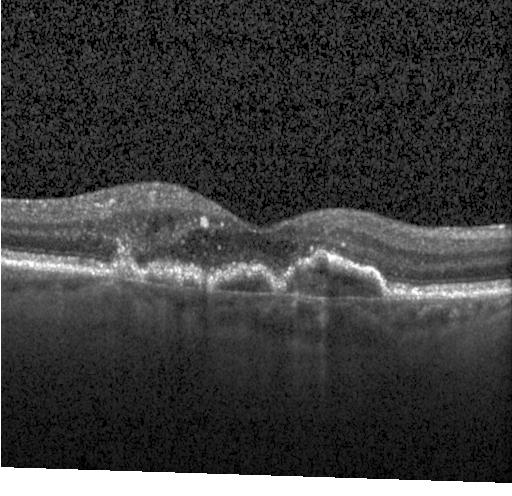 Optical coherence tomography B-scan.
Macular OCT: CNV.